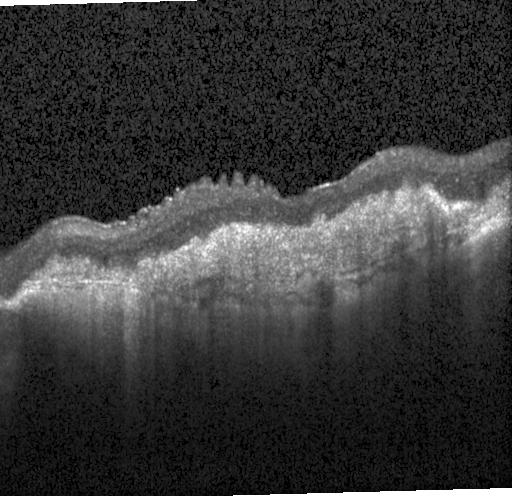

OCT scan showing a choroidal neovascular membrane.